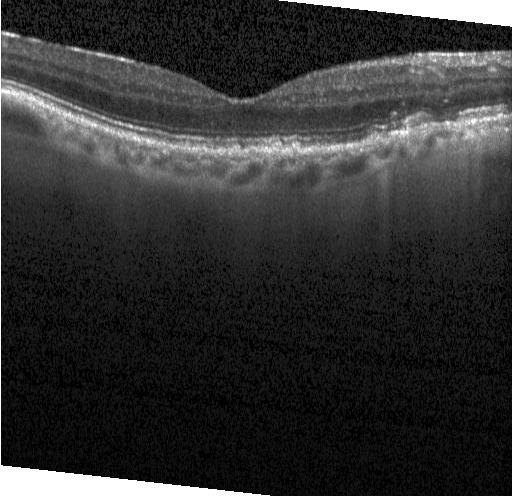 Finding: multiple drusen.